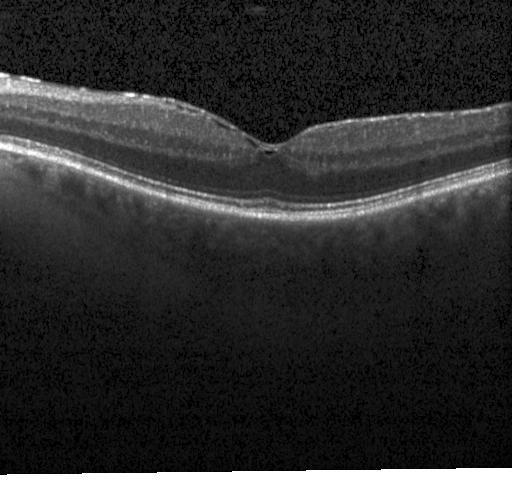
Spectral-domain optical coherence tomography. Macular scan. OCT line scan. Heidelberg Spectralis.
The scan shows no choroidal neovascularization, diabetic macular edema, or drusen.